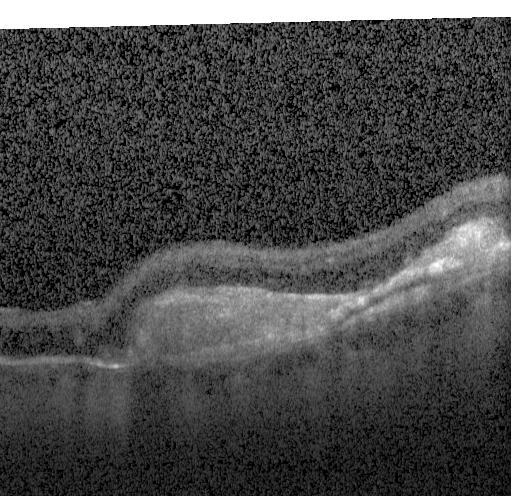
Impression: a choroidal neovascular membrane.